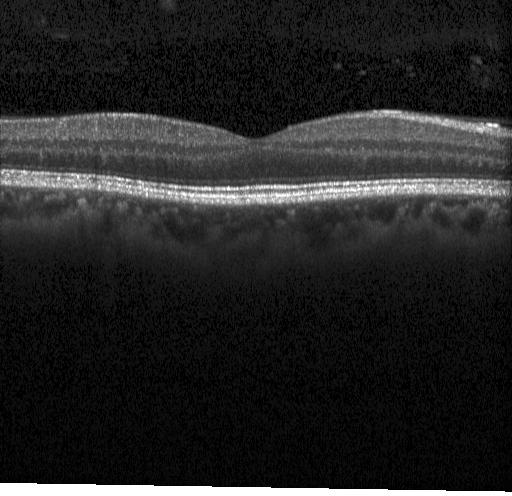
OCT B-scan. Finding: no choroidal neovascularization, diabetic macular edema, or drusen.